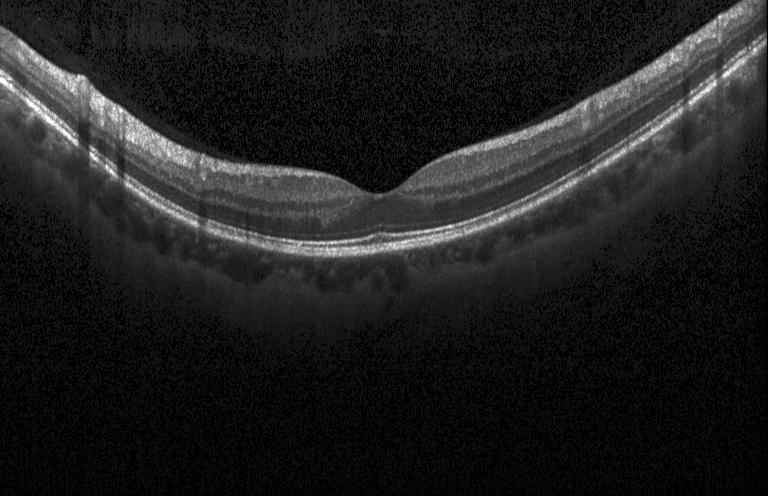

Through the macula, OCT B-scan, Heidelberg Spectralis.
OCT finding: neither choroidal neovascularization, diabetic macular edema, nor drusen.